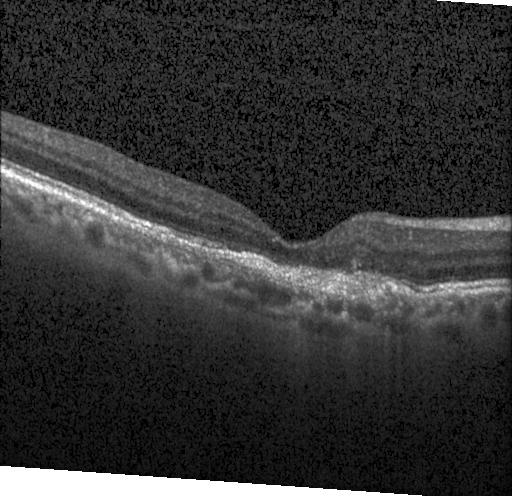
The scan shows a choroidal neovascular membrane.